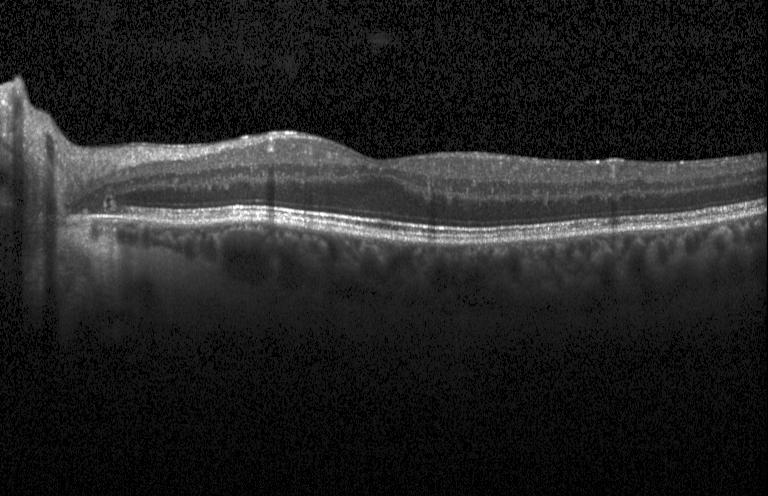

Horizontal scan through the fovea; retinal OCT B-scan.
Diagnosis: neither CNV, DME, nor drusen.